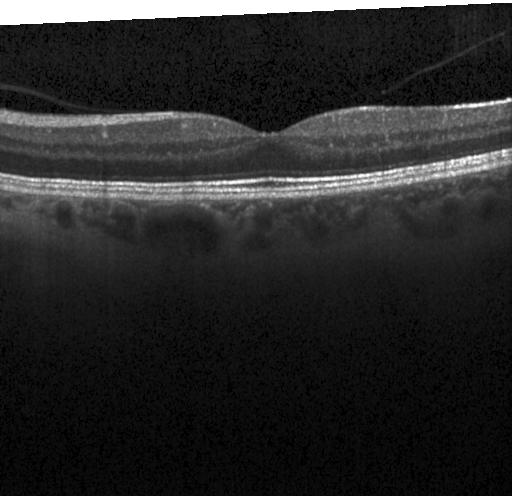

Fovea-centered. Optical coherence tomography scan. Spectral-domain optical coherence tomography — The scan shows no evidence of choroidal neovascularization, diabetic macular edema, or drusen.